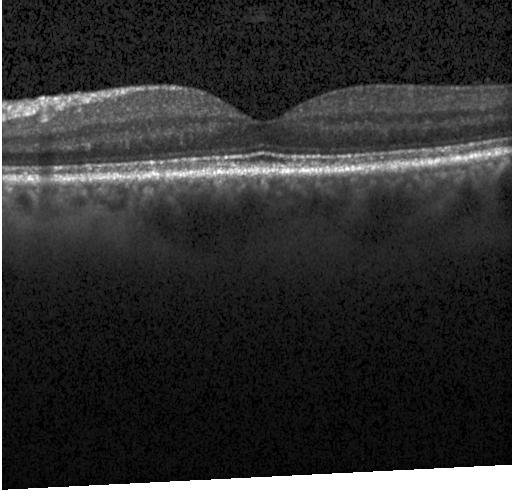 Optical coherence tomography scan · spectral-domain optical coherence tomography · Heidelberg Spectralis · macular scan. This B-scan demonstrates no choroidal neovascularization, diabetic macular edema, or drusen.